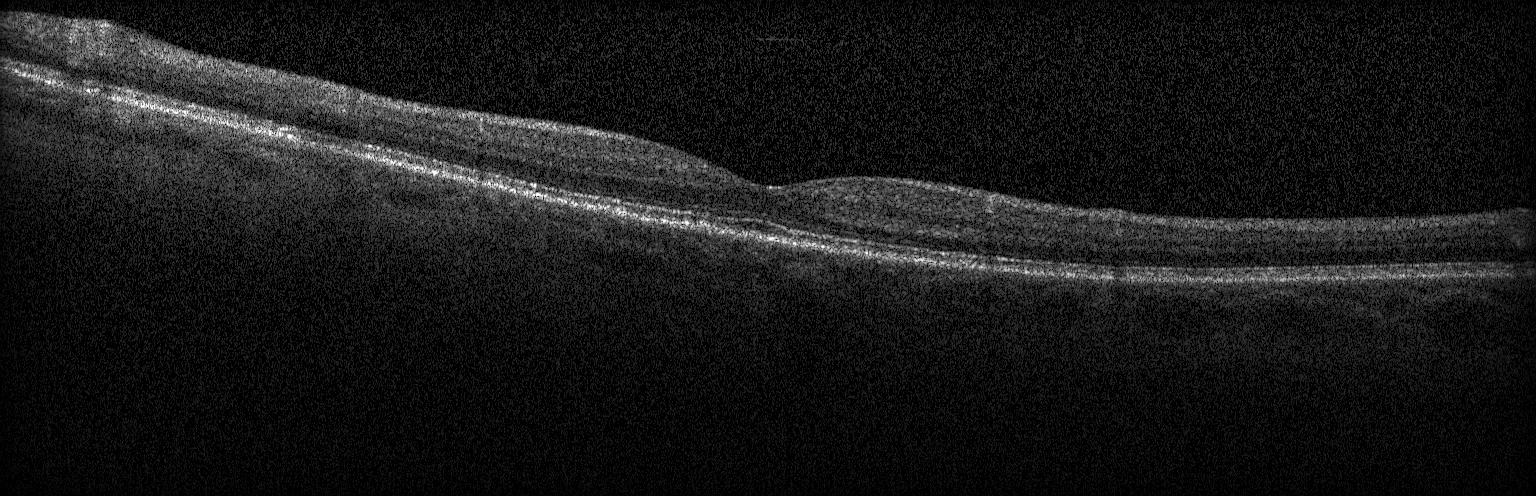
Retinal OCT cross-section. SD-OCT.
Dx: neither CNV, DME, nor drusen.